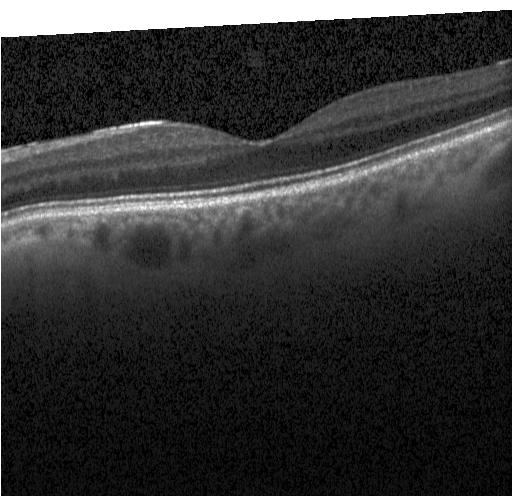
Finding: no choroidal neovascularization, diabetic macular edema, or drusen.